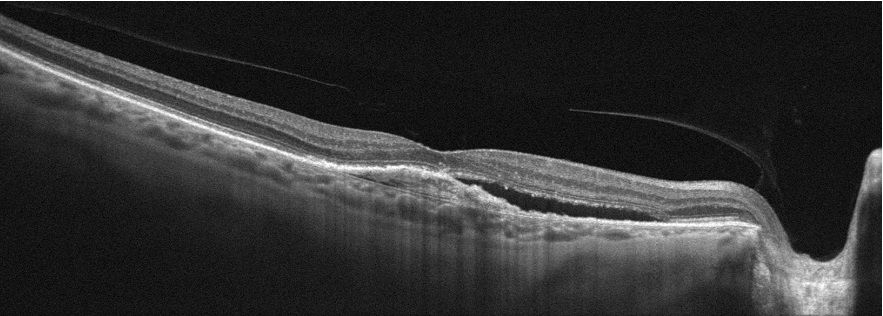

Acquired on an Optovue Avanti RTVue XR, optical coherence tomography B-scan. Diagnosis: AMD.